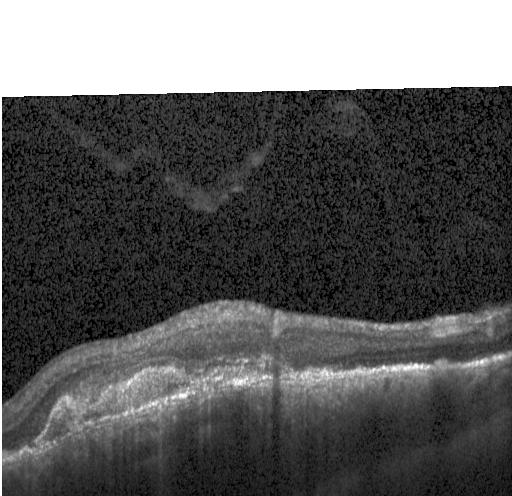 Finding: a choroidal neovascular membrane.